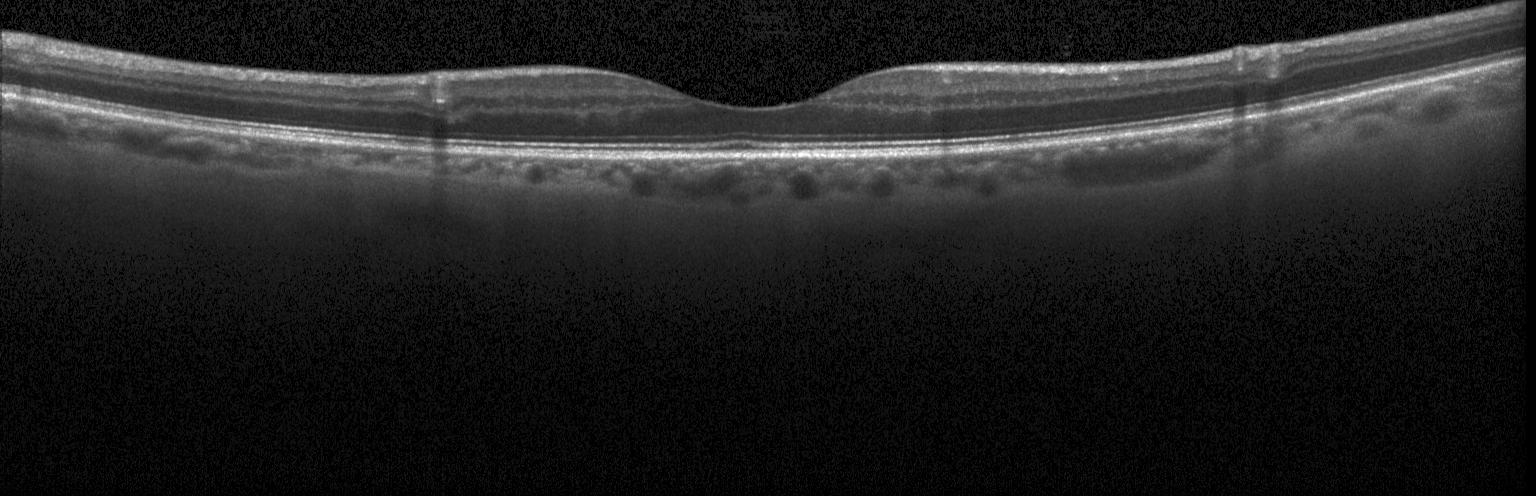 Optical coherence tomography scan · fovea-centered · instrument: Heidelberg Spectralis — This B-scan demonstrates no CNV, no DME, and no drusen.